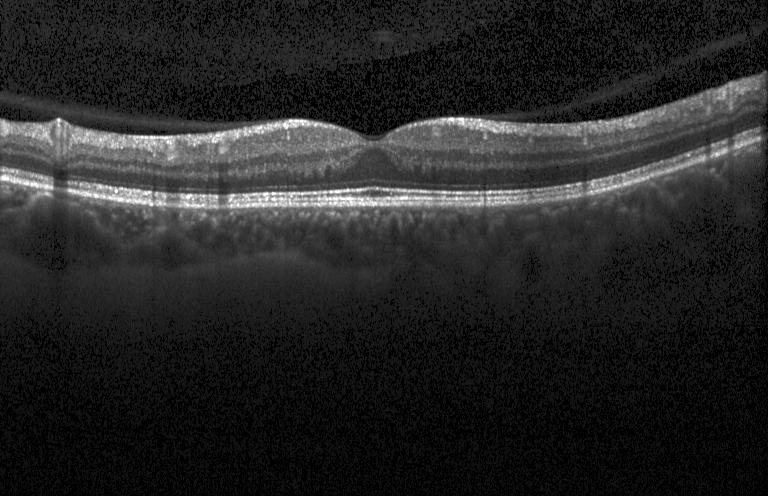
Optical coherence tomography scan · spectral-domain optical coherence tomography.
Macular OCT: no evidence of choroidal neovascularization, diabetic macular edema, or drusen.